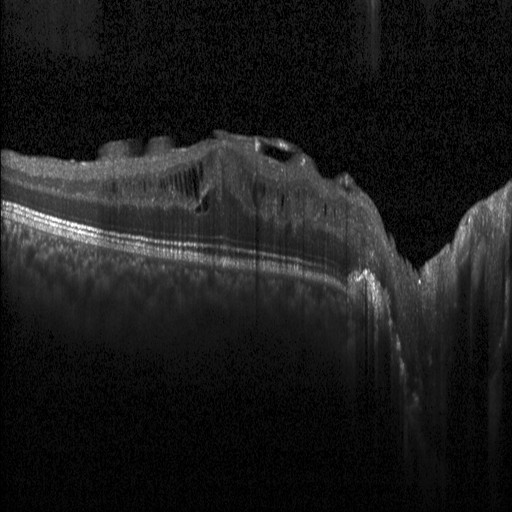 OCT B-scan showing diabetic macular edema.